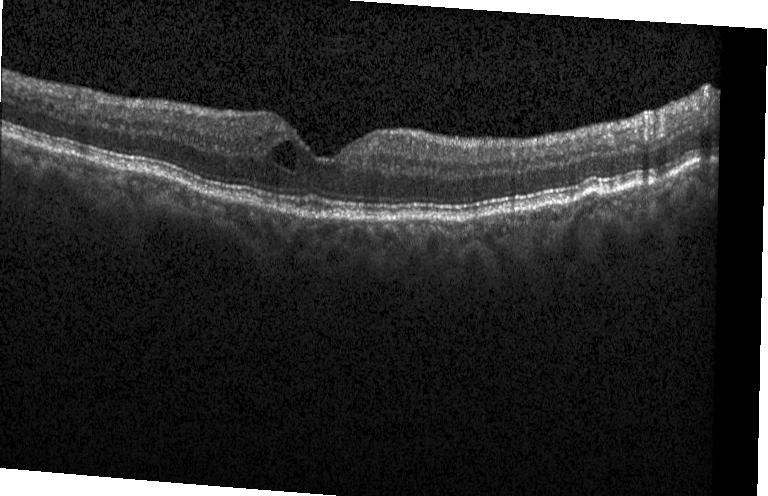
Dx: DME.